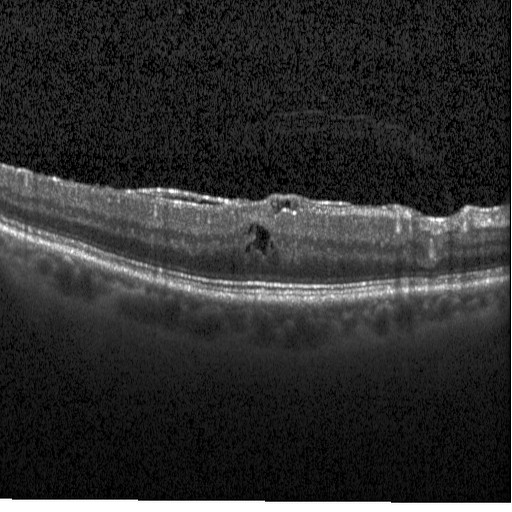

Optical coherence tomography B-scan — Assessment: diabetic macular edema (DME).